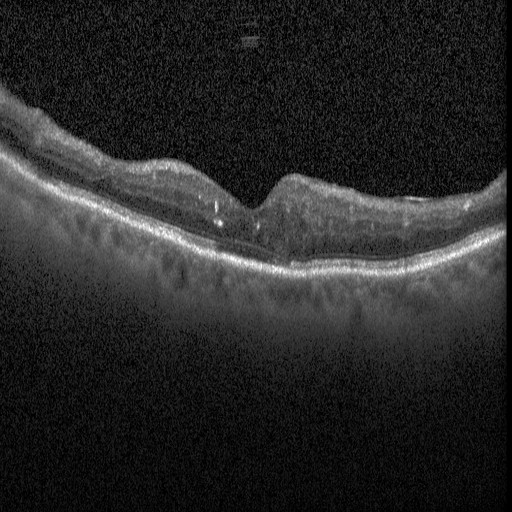 The scan shows diabetic macular edema (DME).